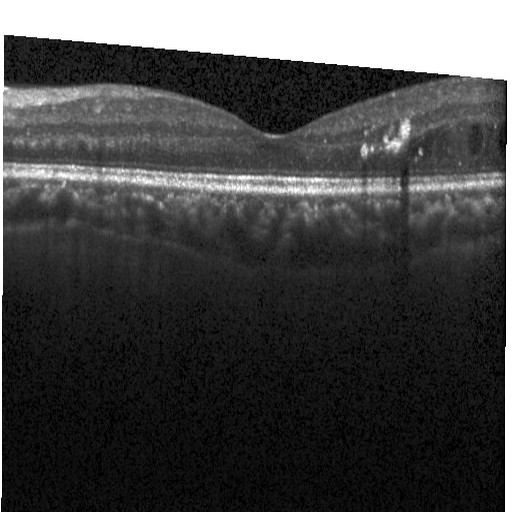

Macular OCT: DME.